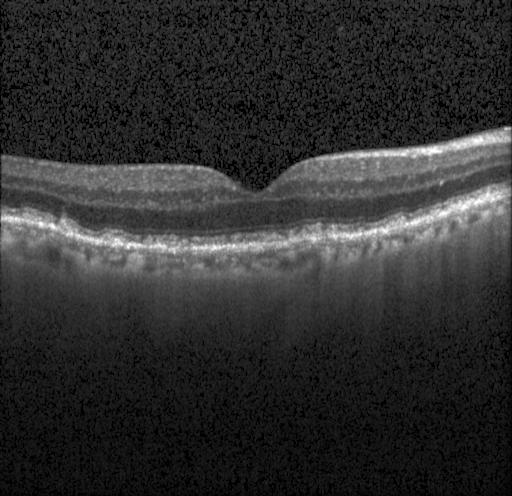
OCT B-scan showing sub-RPE drusenoid deposits.